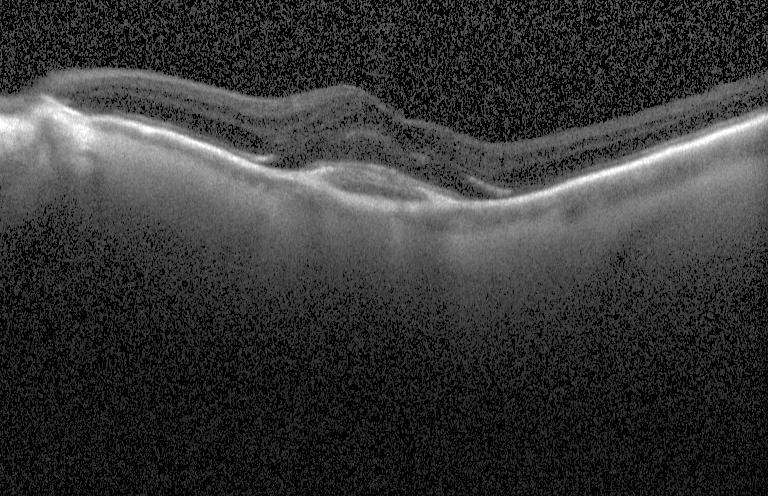

Impression: choroidal neovascularization.